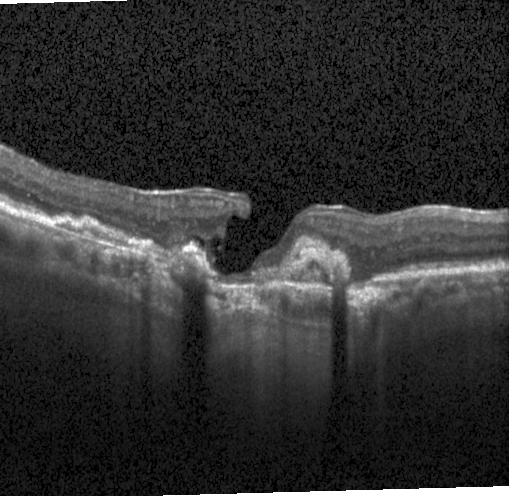
OCT line scan. Impression: a choroidal neovascular membrane.